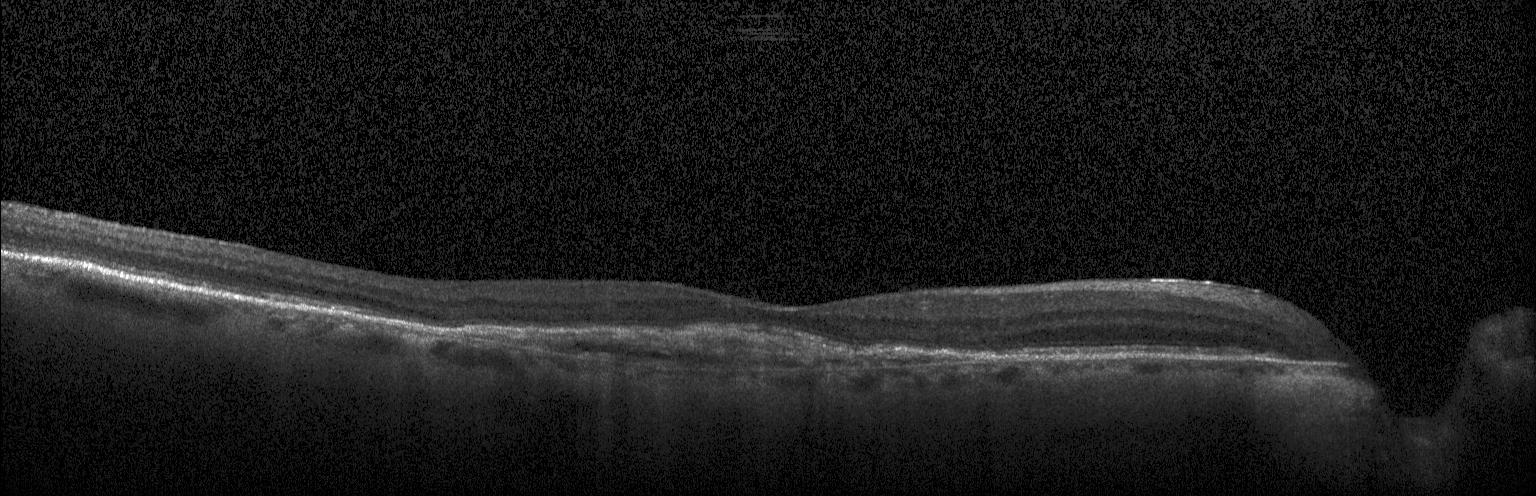
Macular scan, Heidelberg Spectralis OCT system, optical coherence tomography B-scan, spectral-domain OCT. Macular OCT: choroidal neovascularization (CNV).